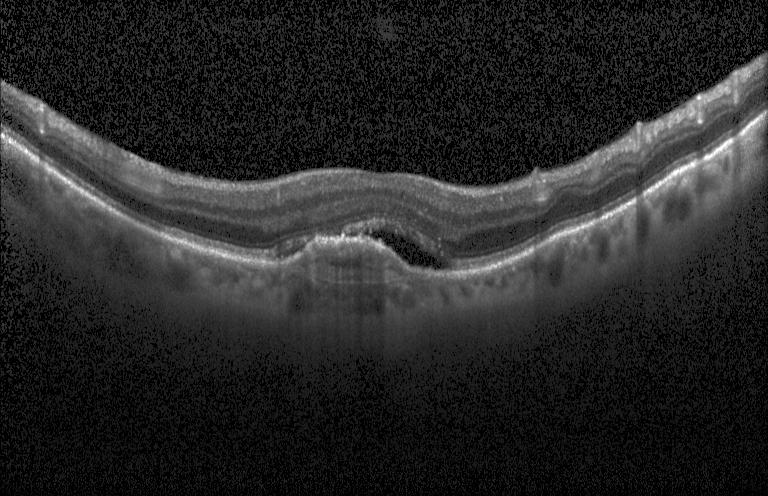
Optical coherence tomography B-scan · centered on the fovea
Macular OCT: choroidal neovascularization.